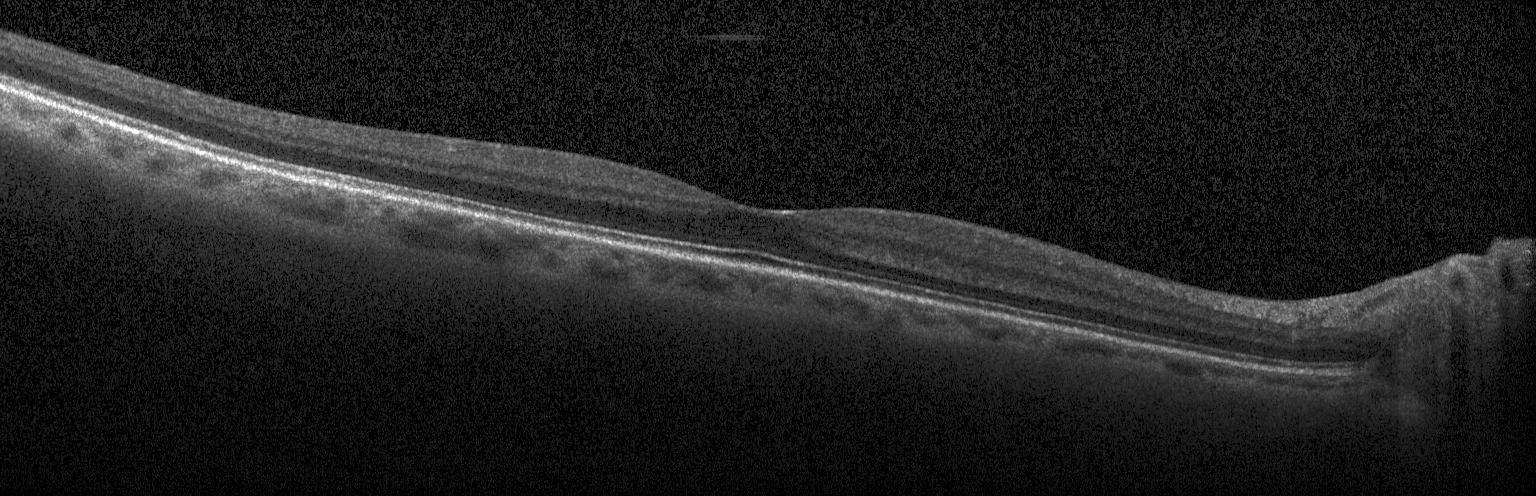 Retinal OCT cross-section; through the macula; spectral-domain optical coherence tomography; Heidelberg Spectralis OCT system.
Diagnosis: no evidence of choroidal neovascularization, diabetic macular edema, or drusen.